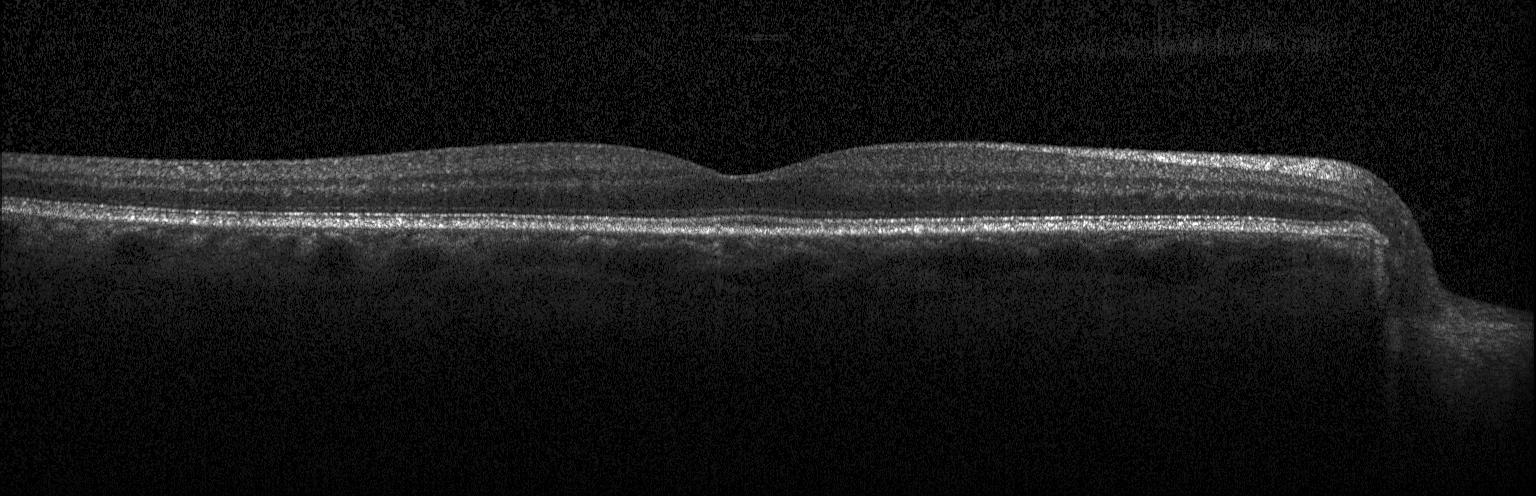
OCT scan showing neither choroidal neovascularization, diabetic macular edema, nor drusen.